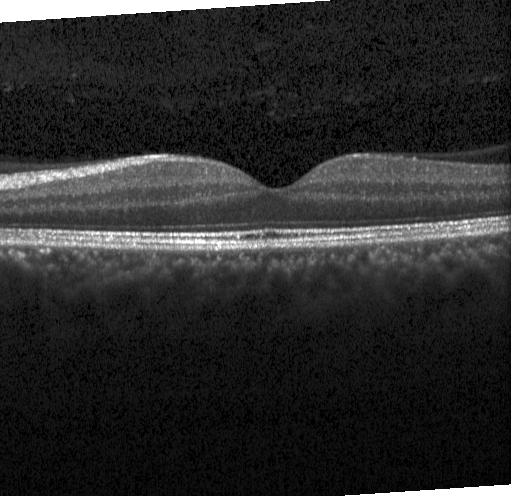 Retinal OCT cross-section showing no evidence of choroidal neovascularization, diabetic macular edema, or drusen.